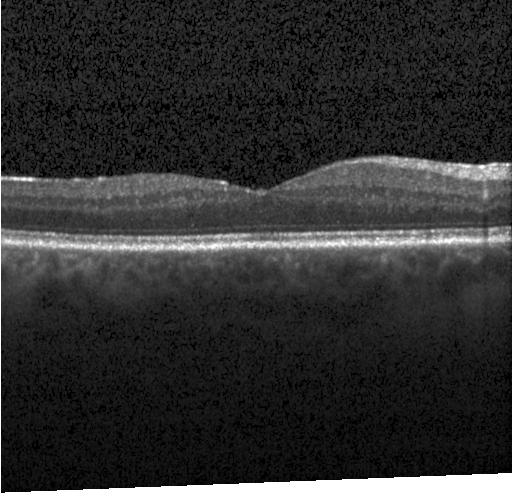

OCT B-scan
No choroidal neovascularization, no diabetic macular edema, and no drusen.